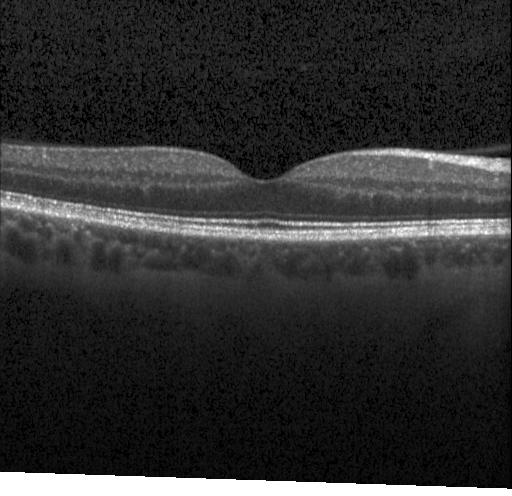 Diagnosis: no choroidal neovascularization, diabetic macular edema, or drusen.